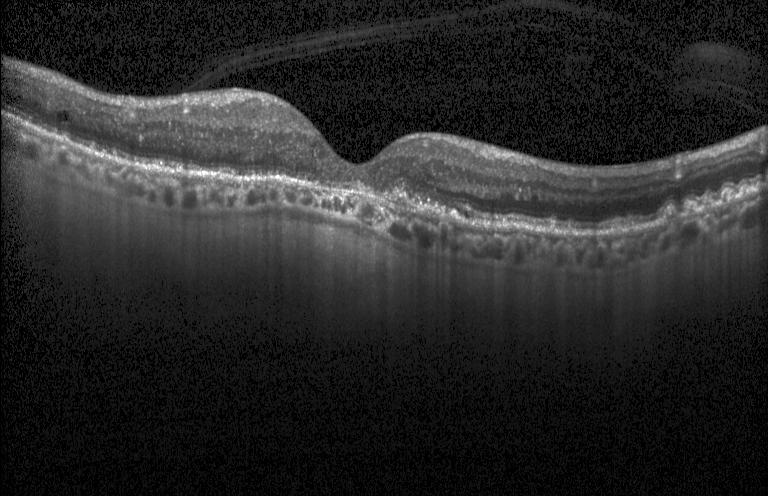
Spectral-domain OCT. OCT line scan. Through the macula. Impression: a choroidal neovascular membrane.